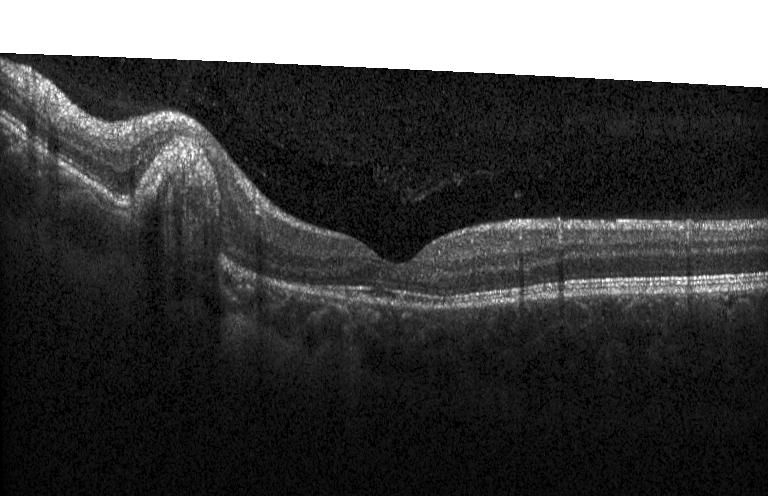

OCT scan showing choroidal neovascularization (CNV).